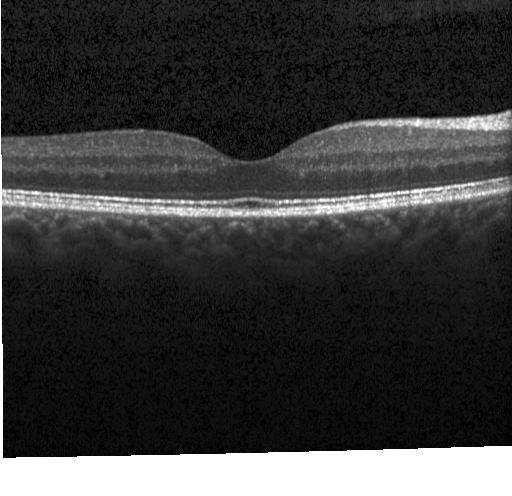
OCT line scan, spectral-domain OCT, instrument: Heidelberg Spectralis. Finding: neither choroidal neovascularization, diabetic macular edema, nor drusen.